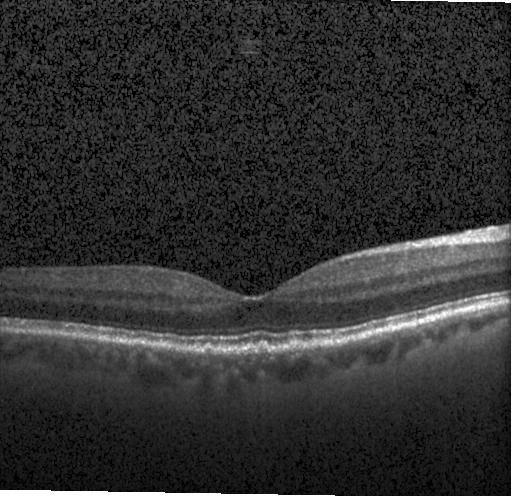
Finding: sub-RPE drusenoid deposits.